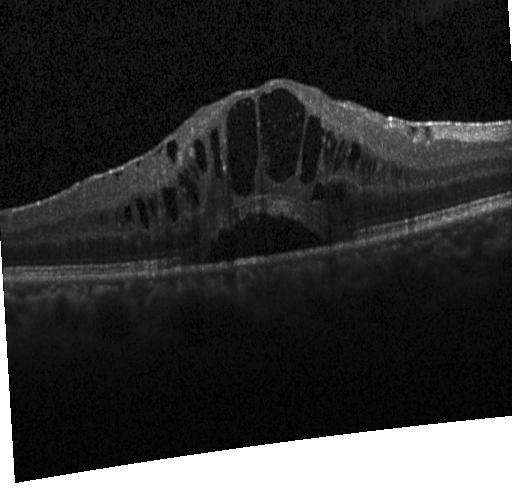 Spectral-domain OCT. OCT B-scan. Fovea-centered. Impression: diabetic macular edema (DME).